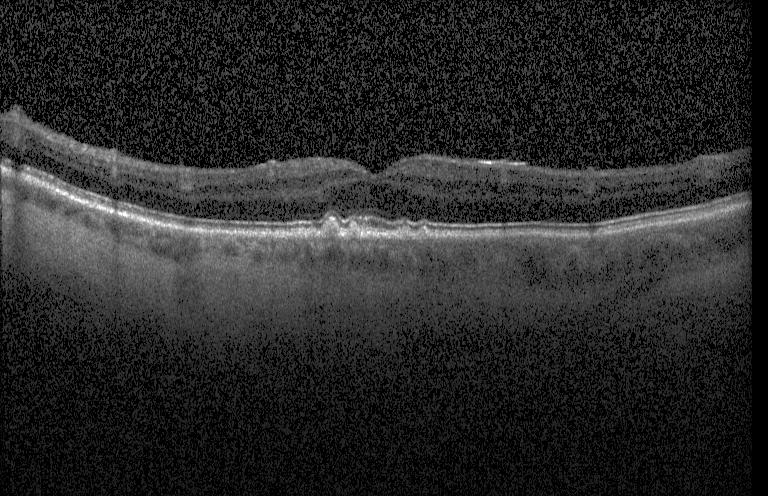 Centered on the fovea · spectral-domain OCT · instrument: Heidelberg Spectralis · retinal OCT cross-section
OCT finding: multiple drusen.